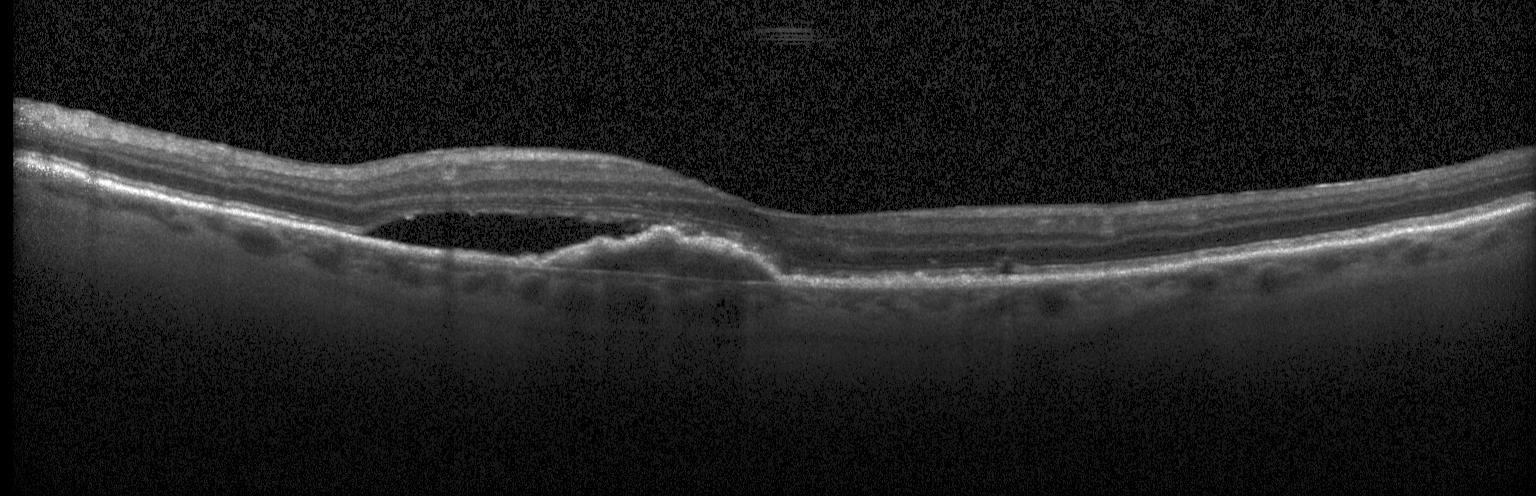 SD-OCT; instrument: Heidelberg Spectralis; OCT line scan. Impression: choroidal neovascularization.